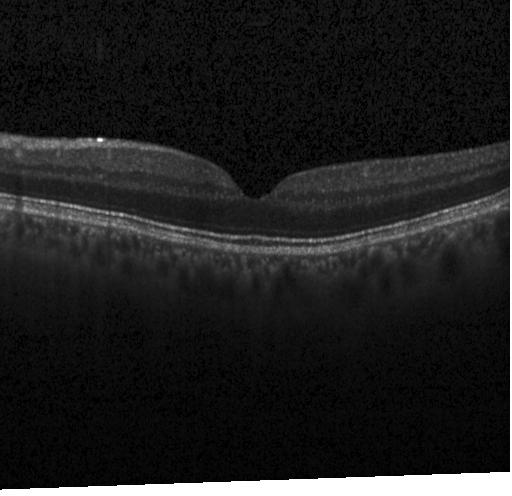

Finding: neither choroidal neovascularization, diabetic macular edema, nor drusen.